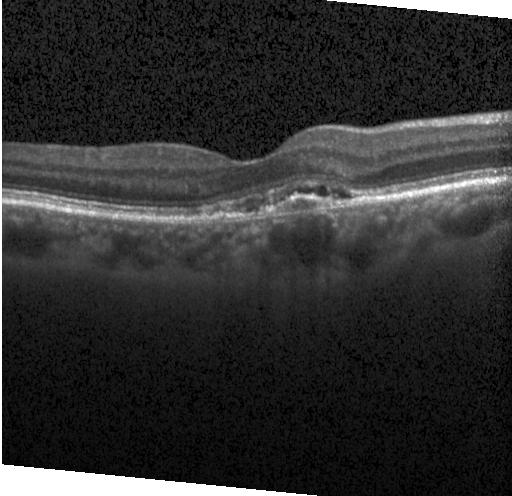

Heidelberg Spectralis OCT system. Retinal OCT cross-section. Through the macula
Assessment: a choroidal neovascular membrane.